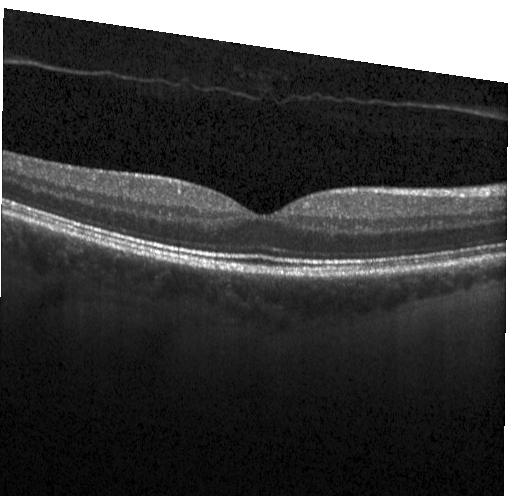
Impression: no evidence of CNV, DME, or drusen.